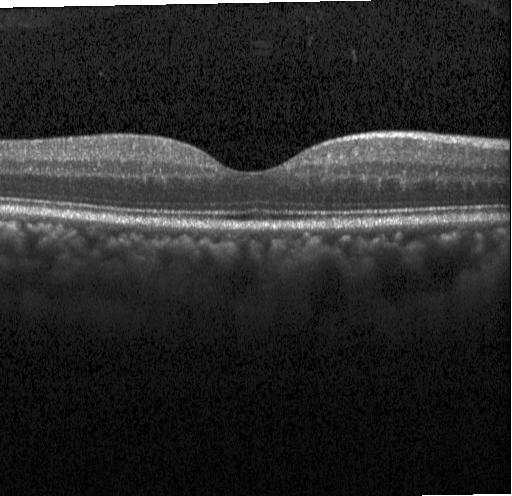
The scan shows no evidence of choroidal neovascularization, diabetic macular edema, or drusen.